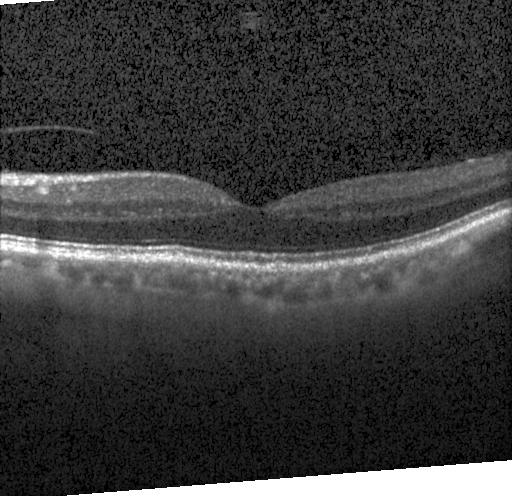

Retinal OCT cross-section; instrument: Heidelberg Spectralis.
Diagnosis: no evidence of choroidal neovascularization, diabetic macular edema, or drusen.